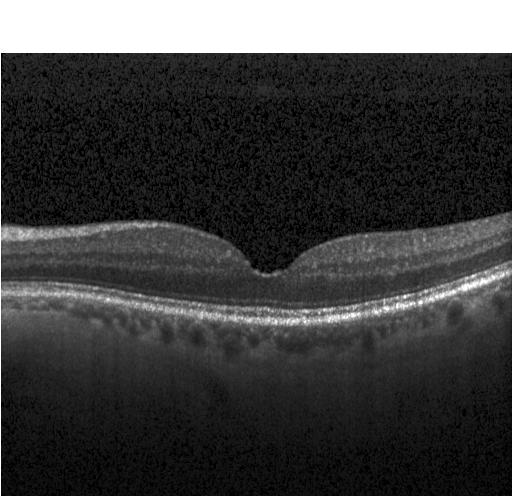 Fovea-centered; Heidelberg Spectralis OCT system; optical coherence tomography scan.
No evidence of choroidal neovascularization, diabetic macular edema, or drusen.